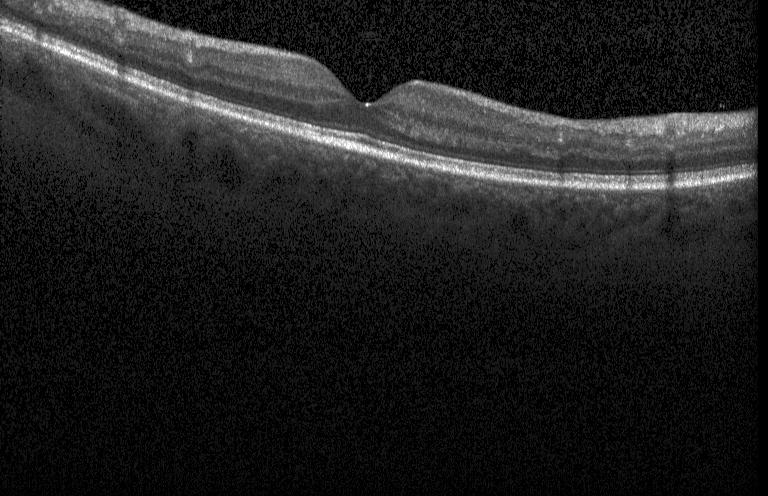
Retinal OCT cross-section showing no choroidal neovascularization, diabetic macular edema, or drusen.